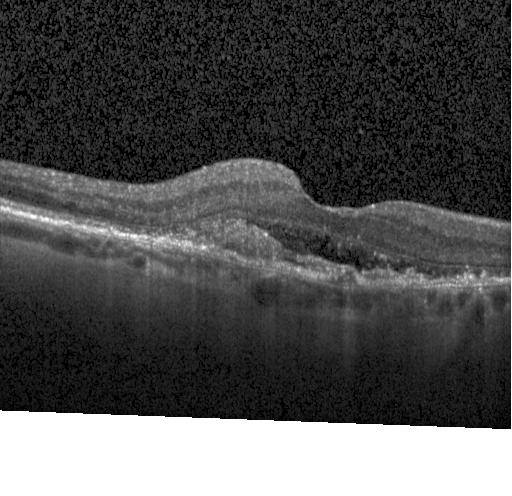

Heidelberg Spectralis OCT system, spectral-domain OCT, retinal OCT cross-section, macular scan.
Dx: a choroidal neovascular membrane.